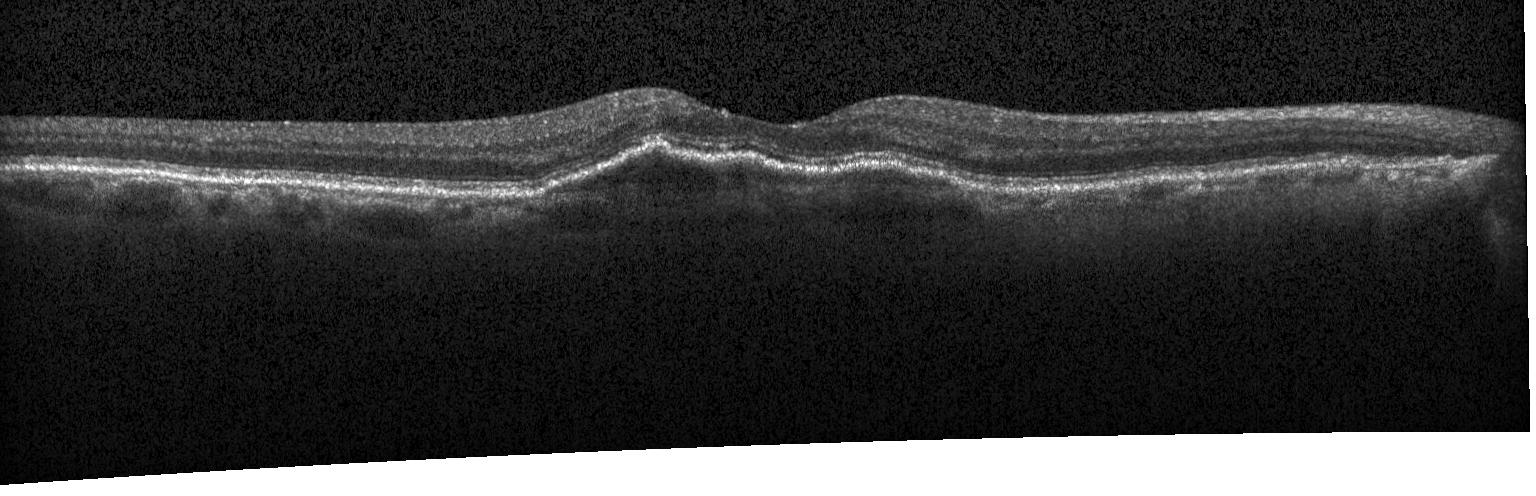

Retinal OCT B-scan
Diagnosis: choroidal neovascularization.